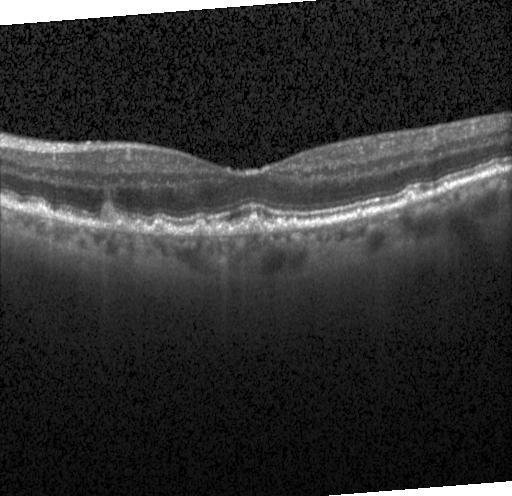

Finding: sub-RPE drusenoid deposits.